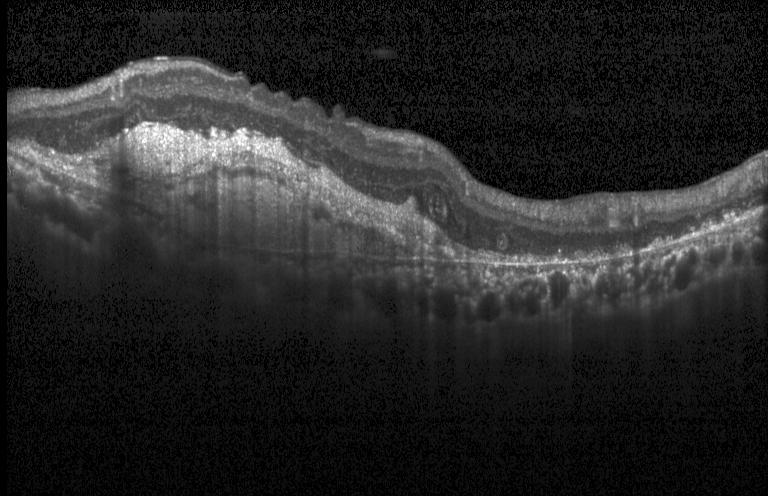
OCT B-scan; horizontal scan through the fovea.
The scan shows choroidal neovascularization (CNV).